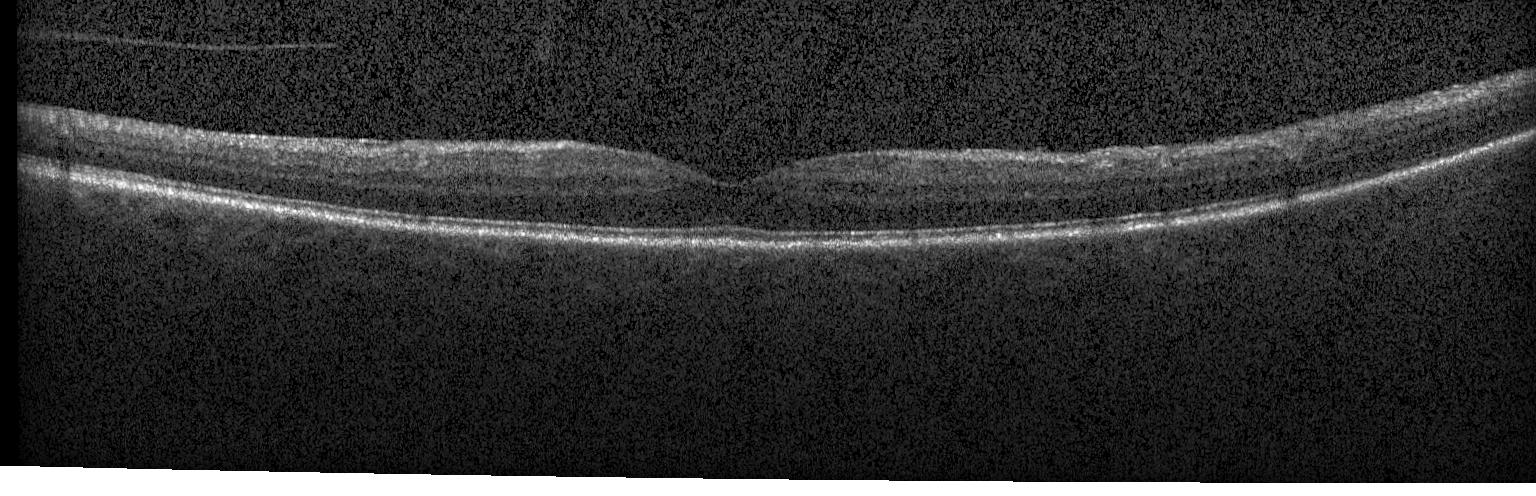

Horizontal scan through the fovea · optical coherence tomography B-scan · Heidelberg Spectralis.
Assessment: no CNV, DME, or drusen.